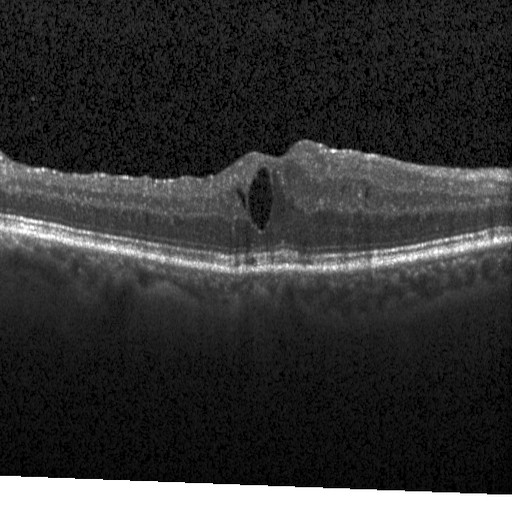
OCT scan showing DME.